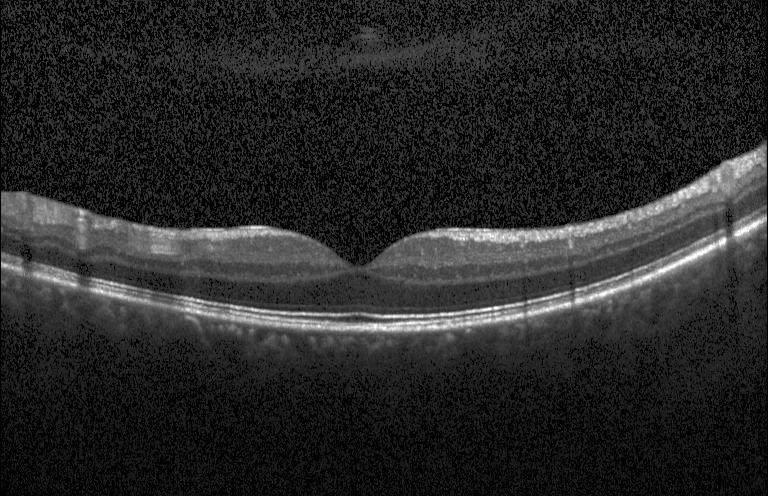 Retinal OCT B-scan
Finding: no evidence of choroidal neovascularization, diabetic macular edema, or drusen.